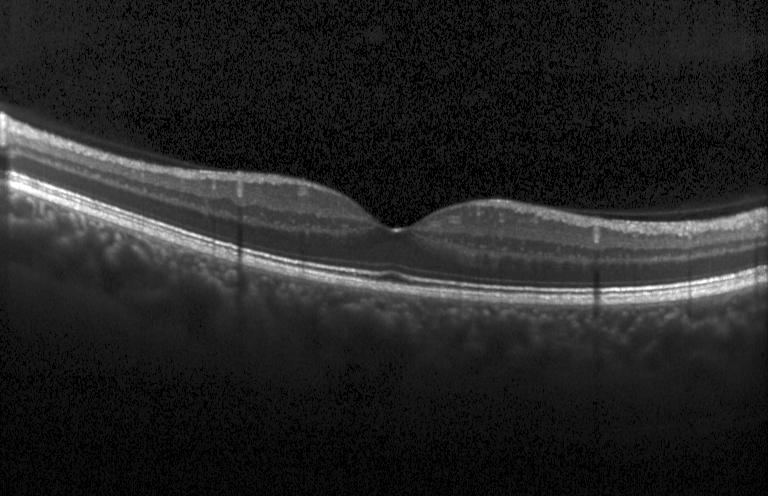

Finding: neither choroidal neovascularization, diabetic macular edema, nor drusen.